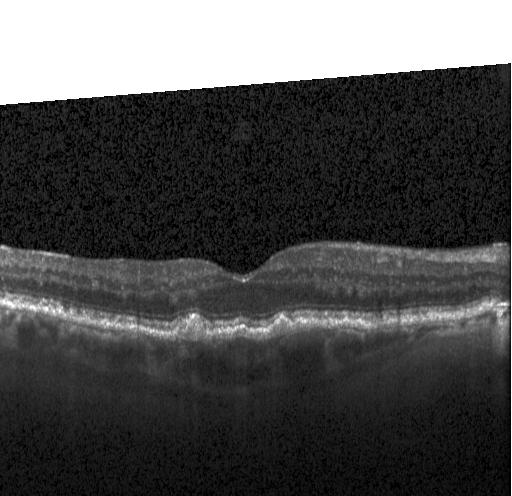

Optical coherence tomography B-scan. Heidelberg Spectralis OCT system. Spectral-domain optical coherence tomography. Horizontal scan through the fovea. Assessment: multiple drusen.